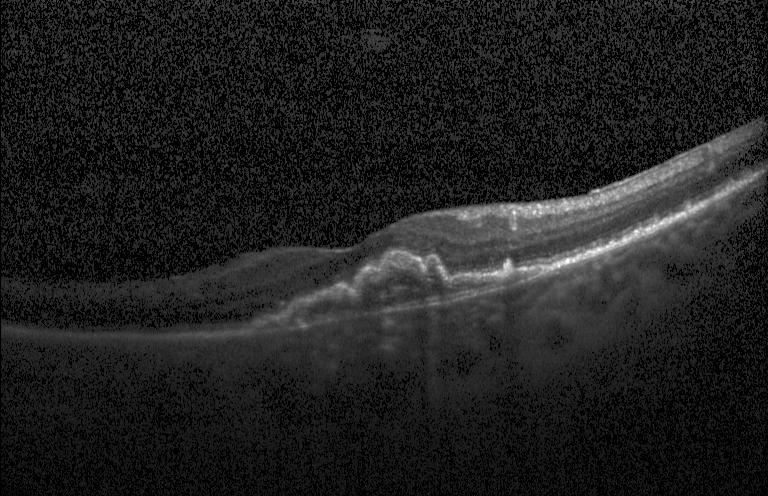
Finding: choroidal neovascularization (CNV).